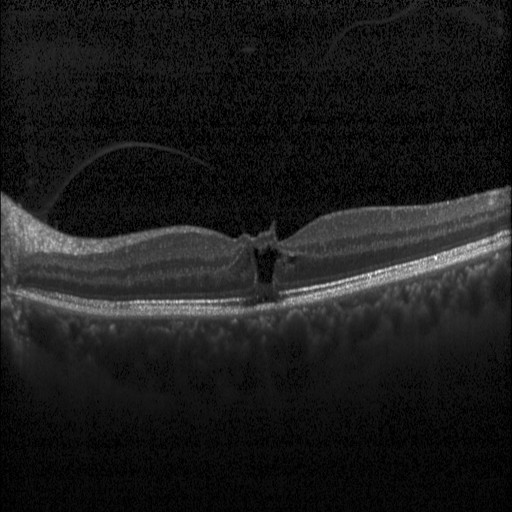 Optical coherence tomography B-scan, Heidelberg Spectralis OCT system.
Finding: diabetic macular edema.